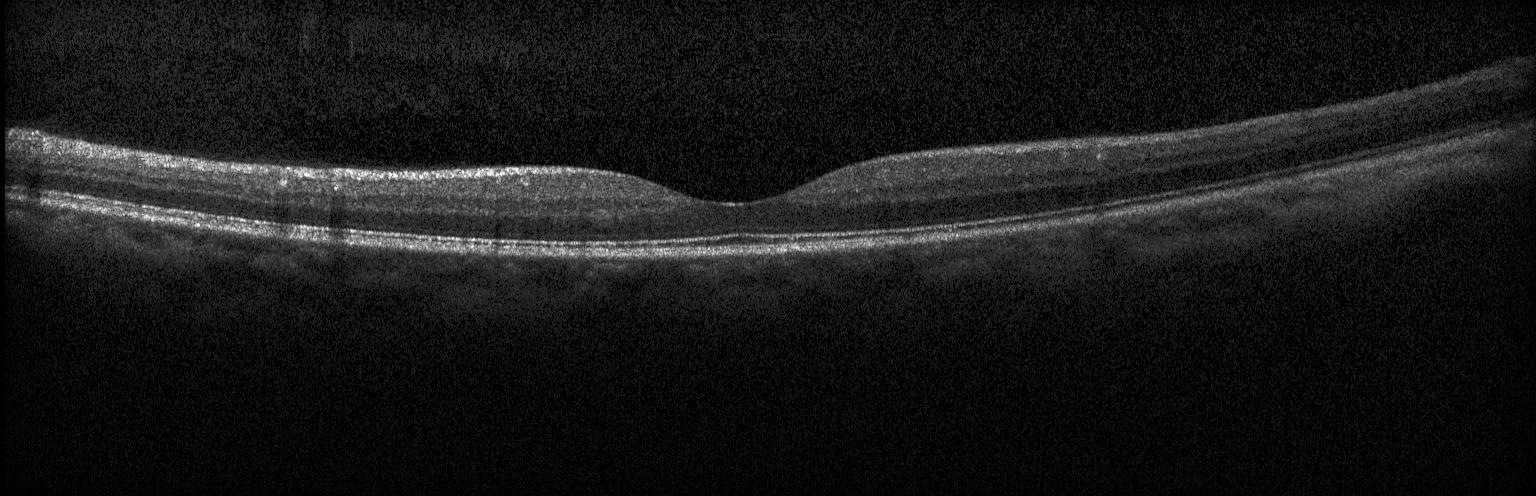

Impression: no evidence of CNV, DME, or drusen.